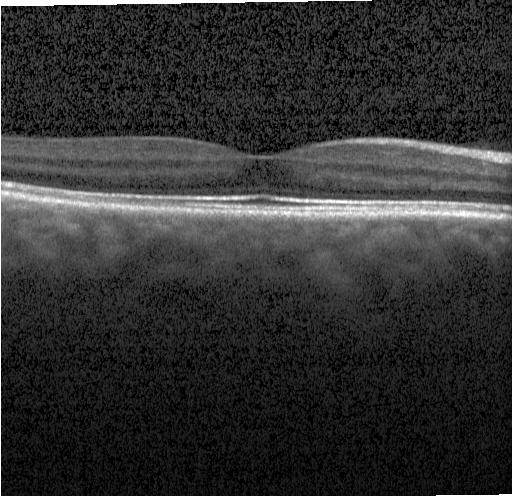
OCT finding: no evidence of CNV, DME, or drusen.